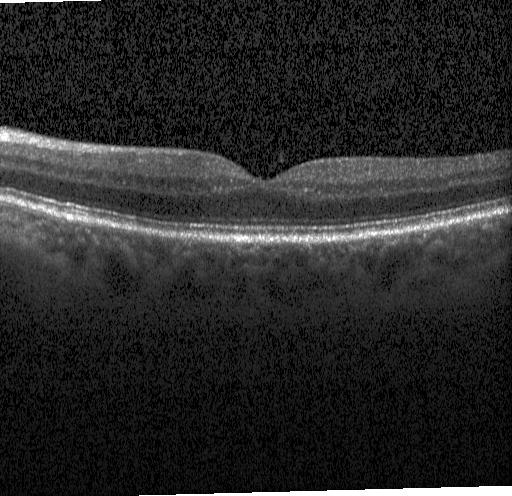

Finding: neither choroidal neovascularization, diabetic macular edema, nor drusen.